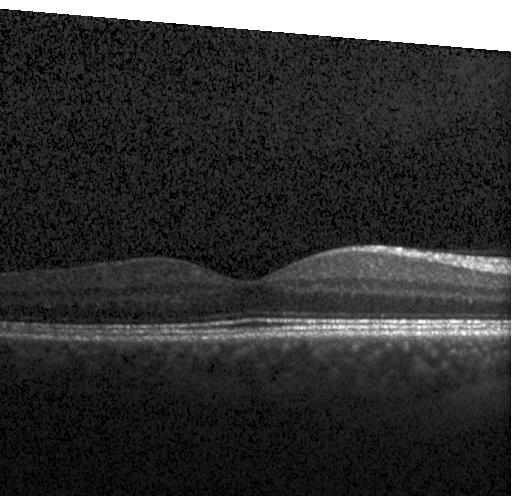

OCT scan showing no evidence of choroidal neovascularization, diabetic macular edema, or drusen.